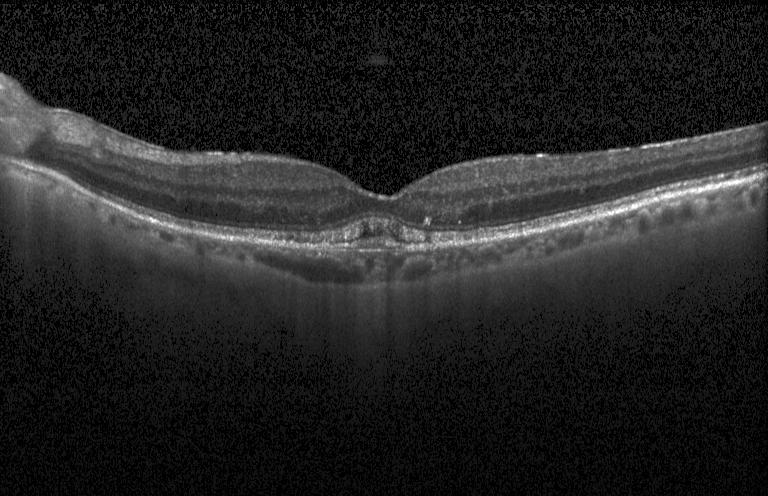 Spectral-domain OCT; optical coherence tomography B-scan
OCT finding: a choroidal neovascular membrane.